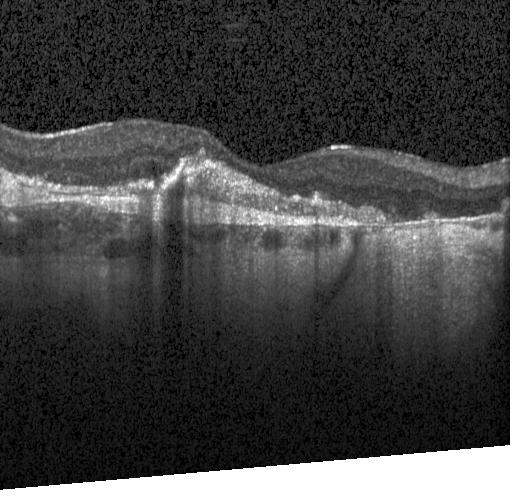

This B-scan demonstrates choroidal neovascularization.